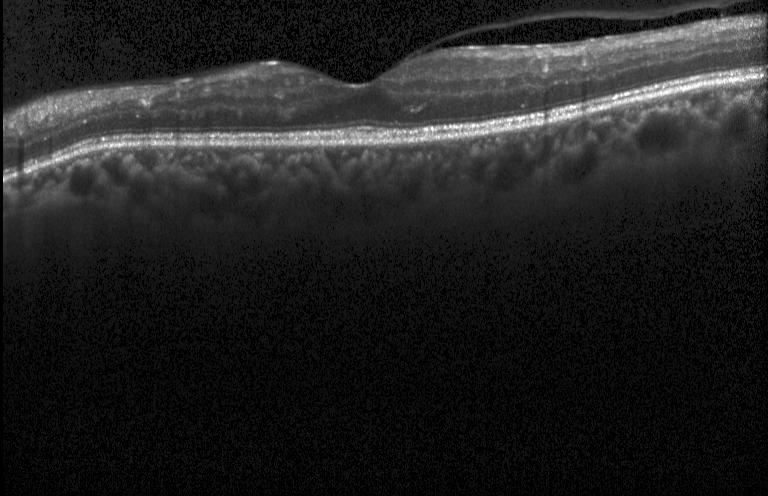 Spectral-domain optical coherence tomography. Instrument: Heidelberg Spectralis. Optical coherence tomography scan. Diabetic macular edema (DME).